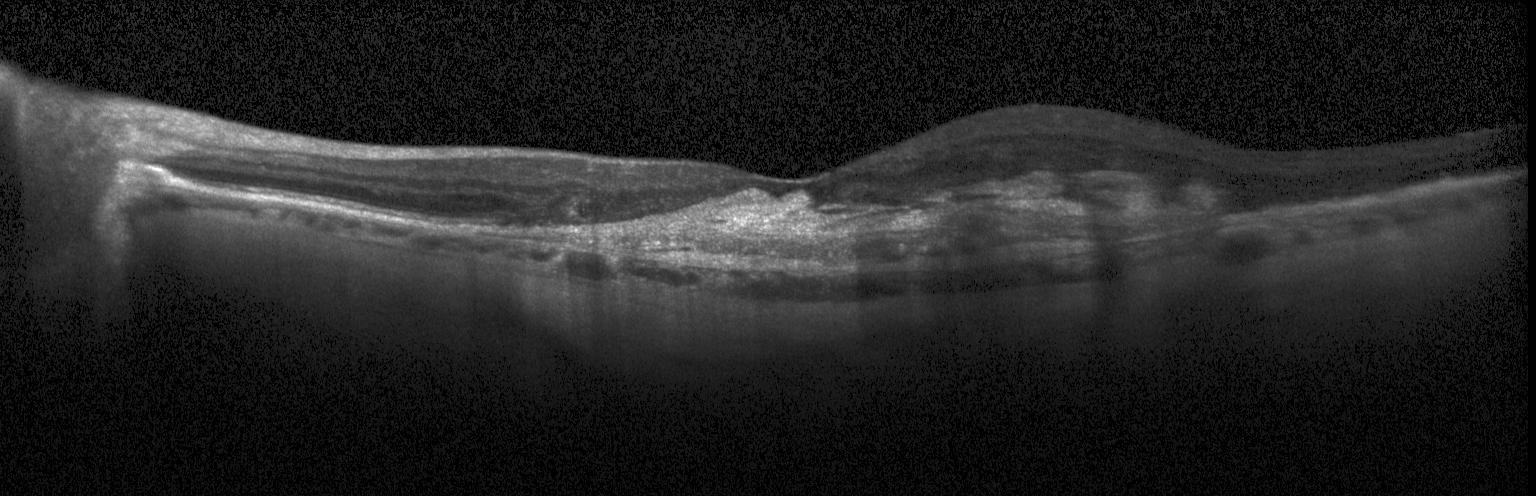 OCT B-scan.
Impression: a choroidal neovascular membrane.